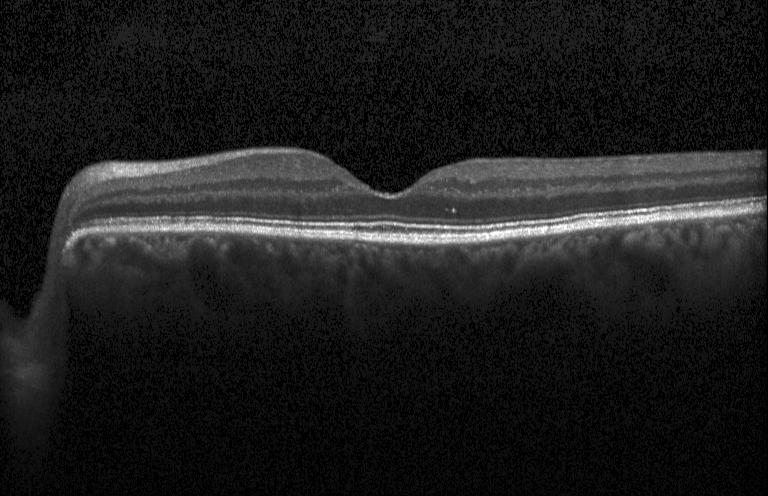

Optical coherence tomography scan; acquired on a Heidelberg Spectralis — Macular OCT: neither CNV, DME, nor drusen.